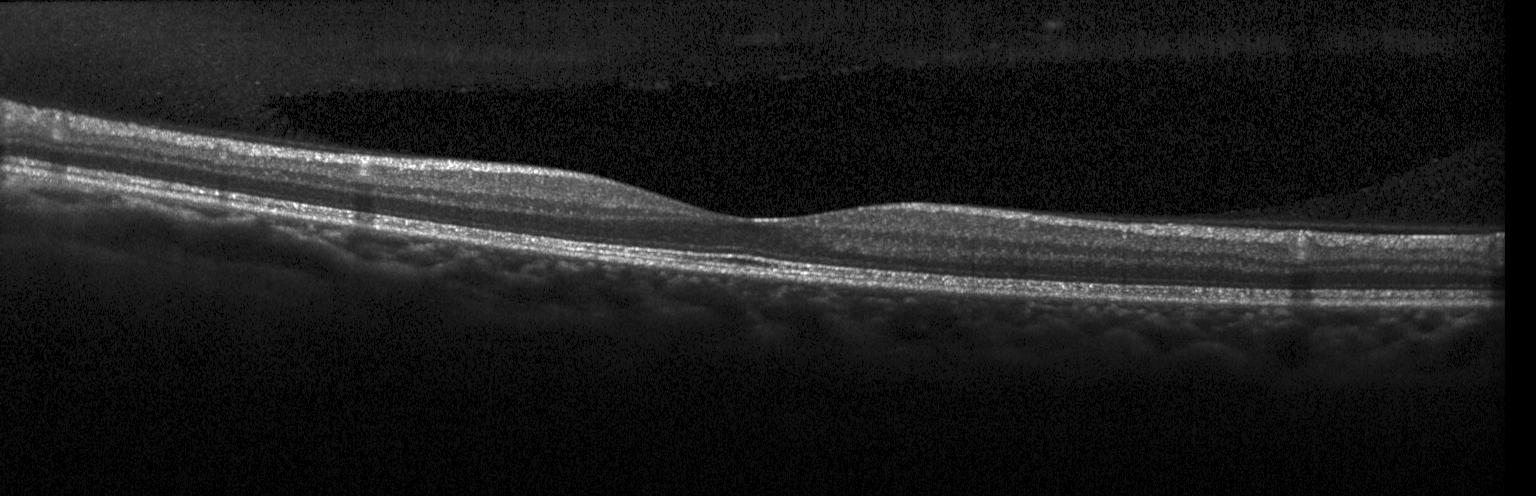 Retinal OCT B-scan. Impression: no evidence of choroidal neovascularization, diabetic macular edema, or drusen.